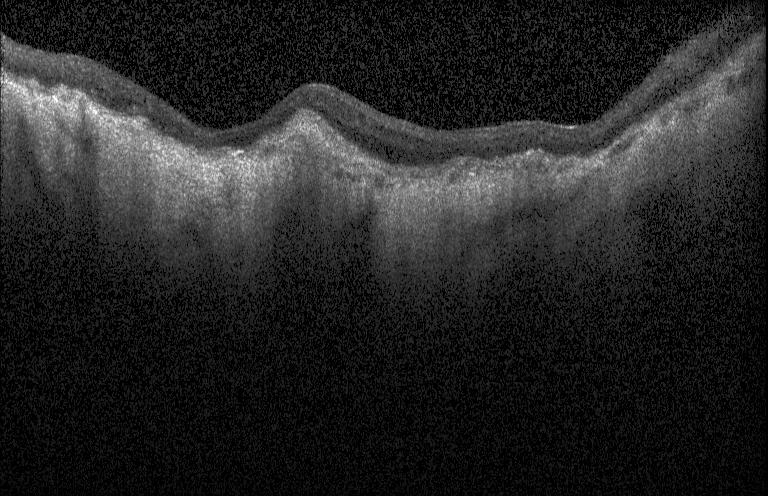

Assessment: choroidal neovascularization (CNV).